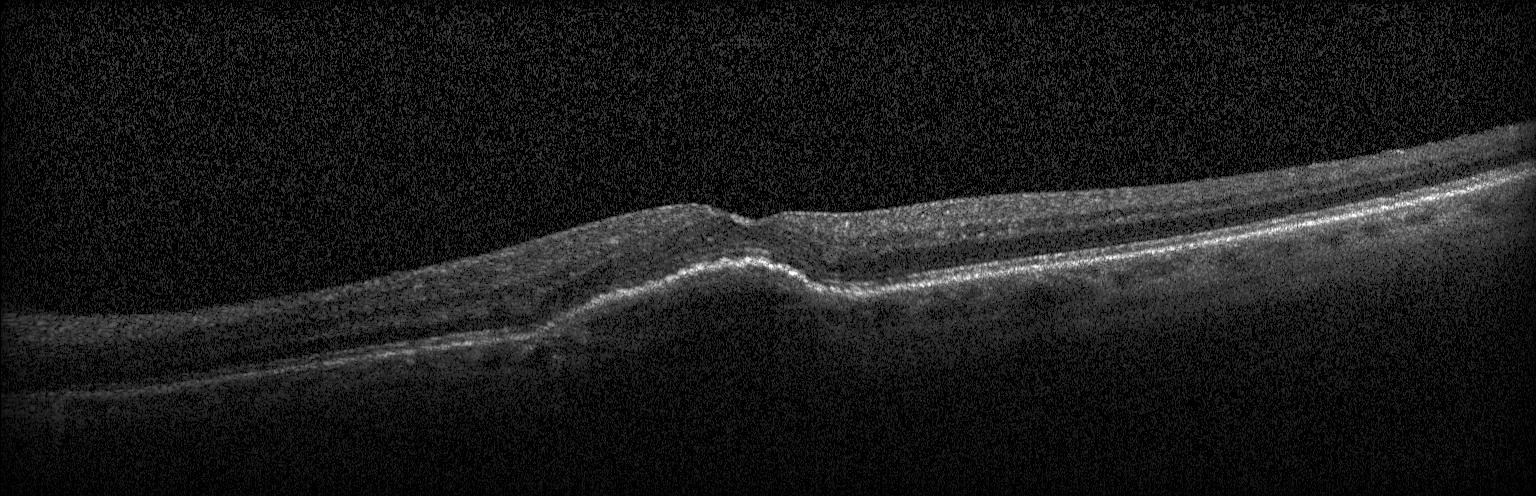 OCT B-scan — Finding: choroidal neovascularization.